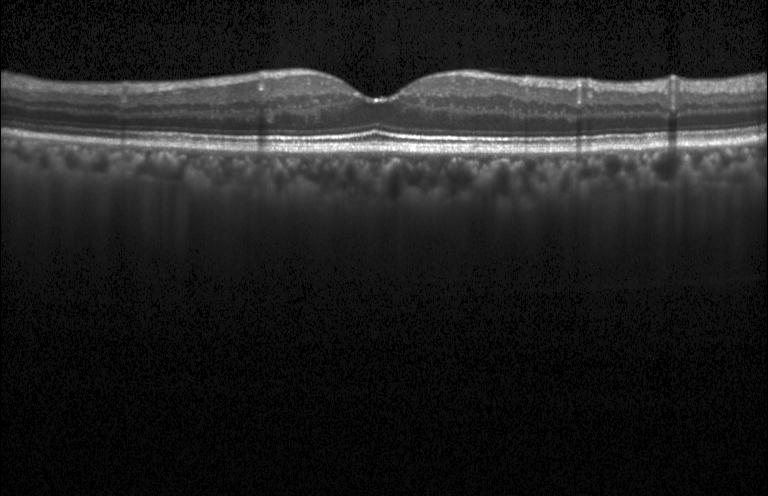

Through the macula · optical coherence tomography scan · Heidelberg Spectralis OCT system — OCT finding: no choroidal neovascularization, diabetic macular edema, or drusen.